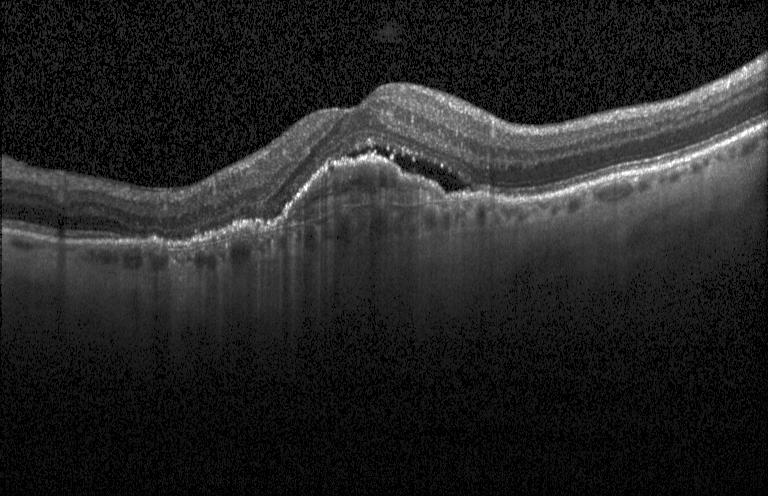 This B-scan demonstrates choroidal neovascularization.